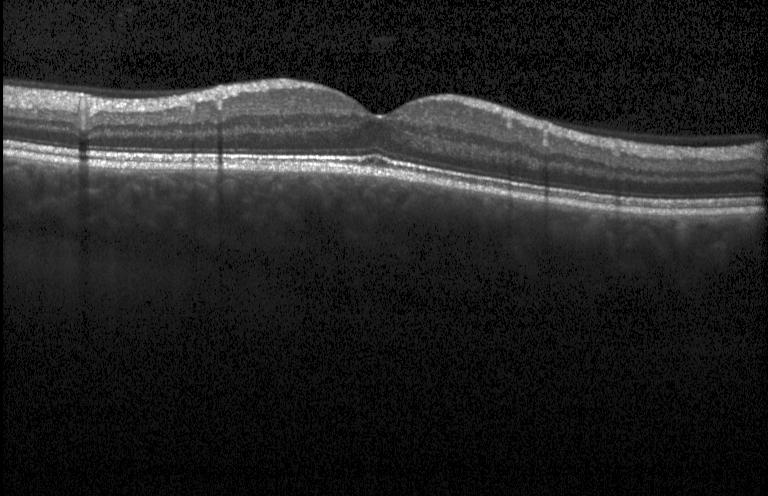
Diagnosis: no choroidal neovascularization, diabetic macular edema, or drusen.